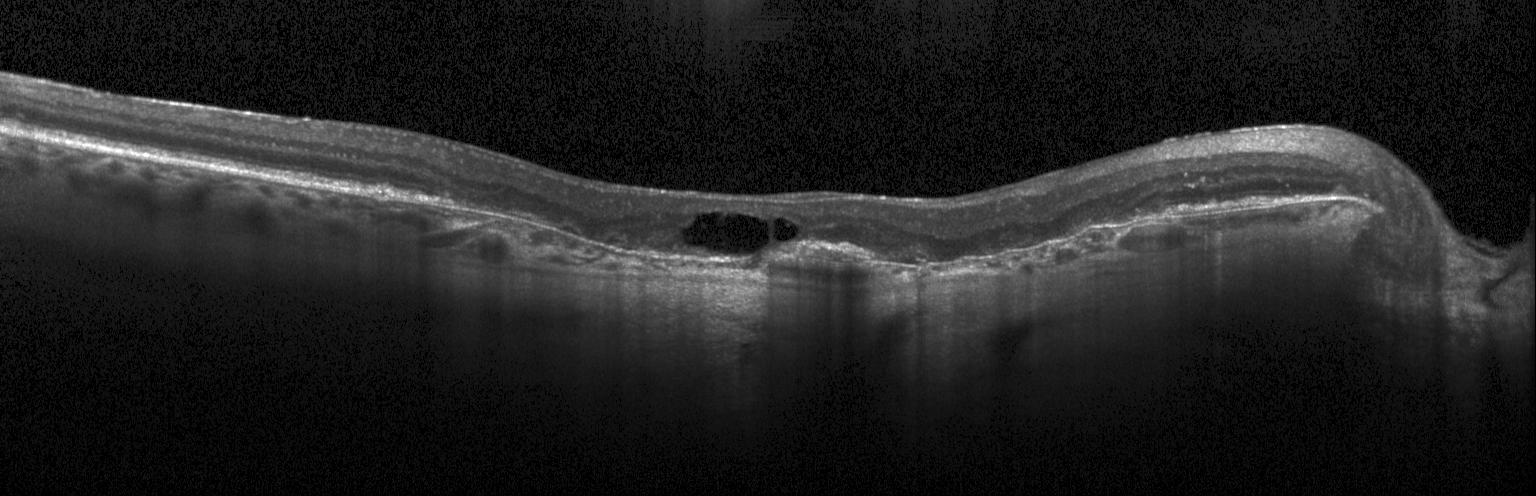
Spectral-domain OCT B-scan: a choroidal neovascular membrane.